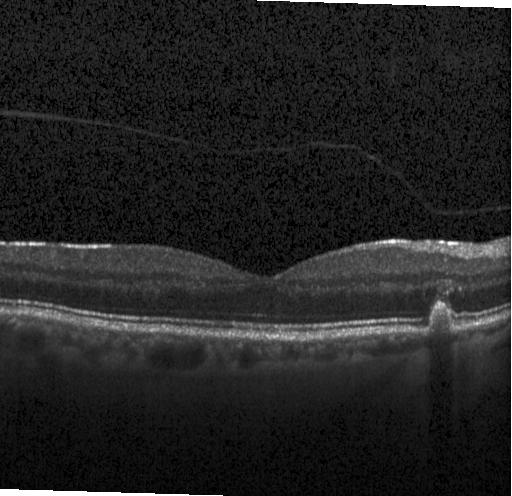

OCT finding: multiple drusen.